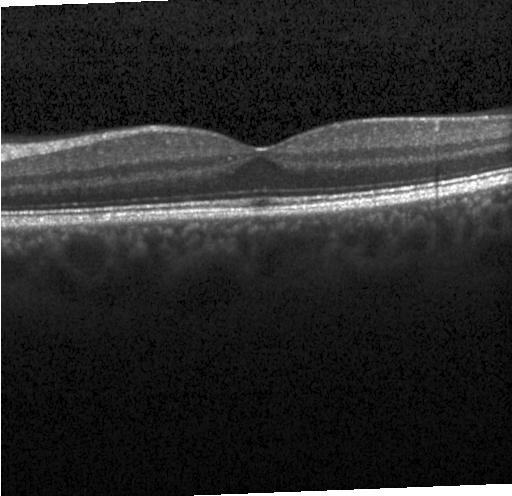 No choroidal neovascularization, no diabetic macular edema, and no drusen.